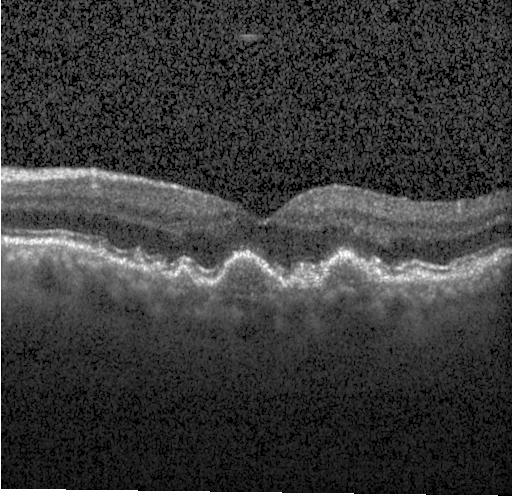
Finding: multiple drusen.